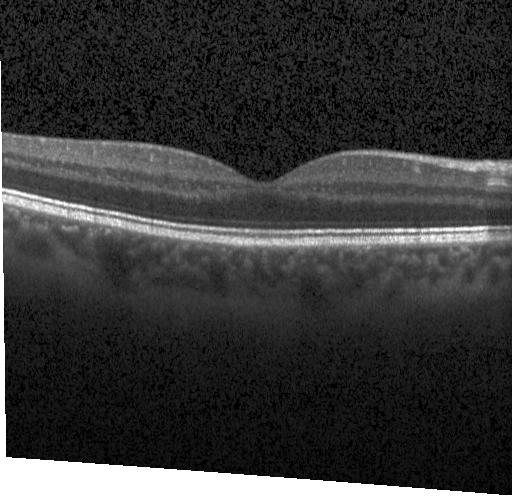

Macular OCT demonstrating no choroidal neovascularization, diabetic macular edema, or drusen.